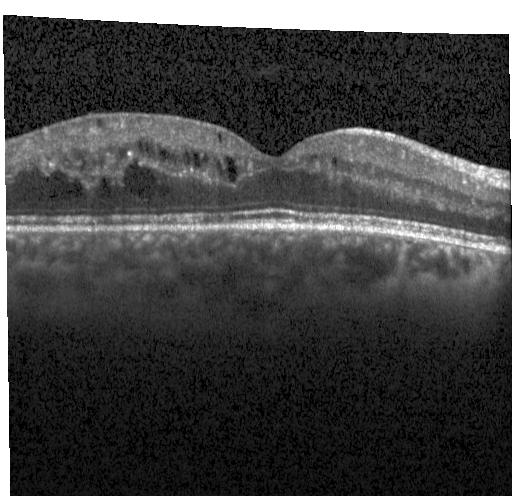

OCT B-scan showing diabetic macular edema.